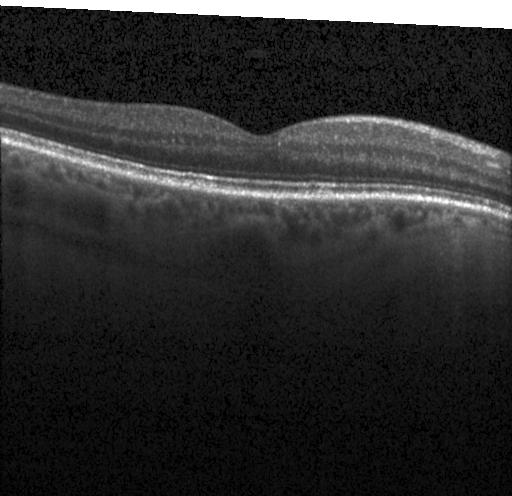
OCT line scan, Heidelberg Spectralis OCT system, spectral-domain OCT, horizontal scan through the fovea — Assessment: no choroidal neovascularization, no diabetic macular edema, and no drusen.